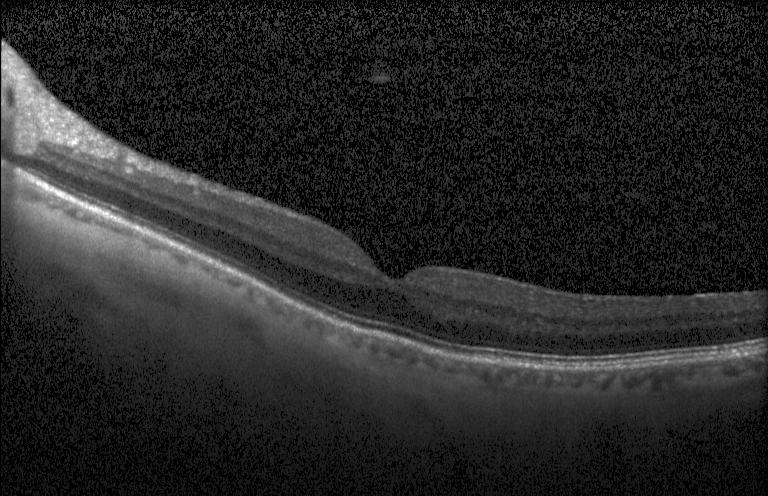

Dx: neither CNV, DME, nor drusen.